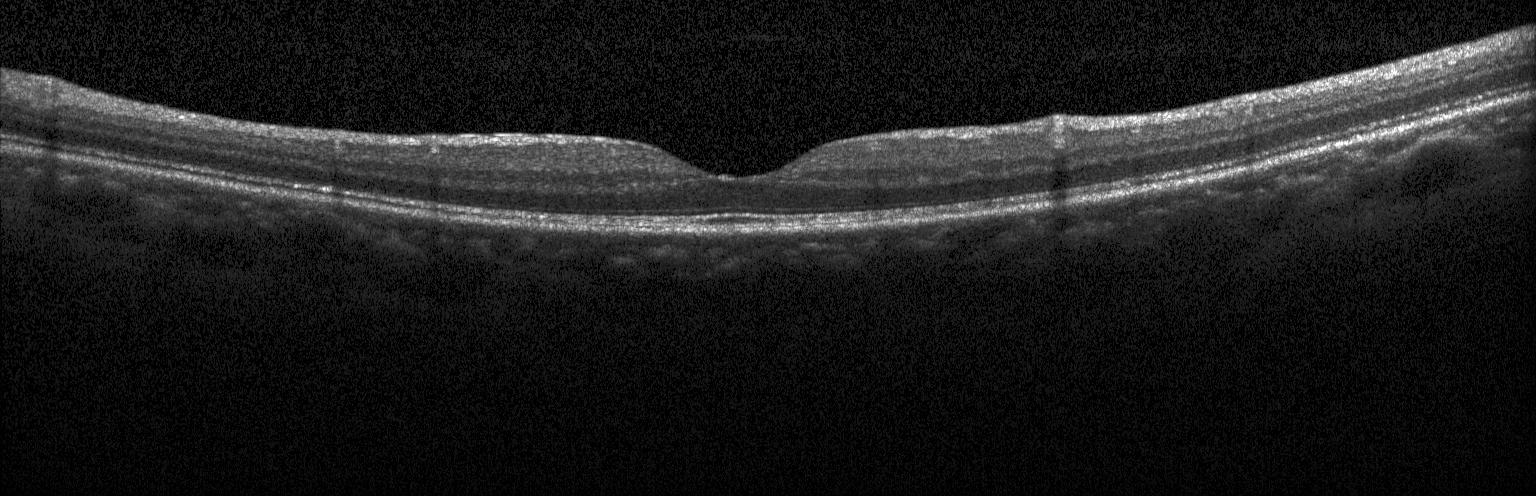 Retinal OCT B-scan; macular scan.
Assessment: no choroidal neovascularization, diabetic macular edema, or drusen.